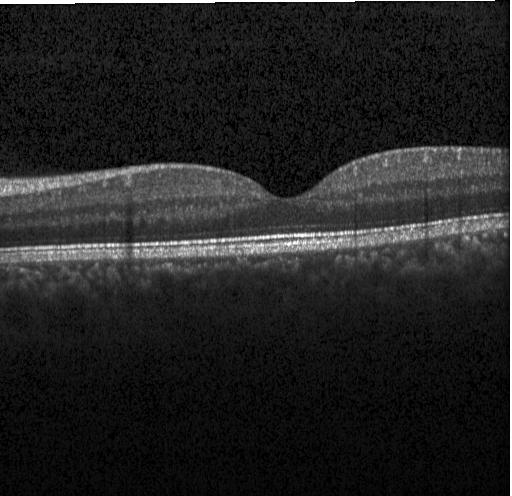

Heidelberg Spectralis OCT system, OCT line scan — Diagnosis: no choroidal neovascularization, no diabetic macular edema, and no drusen.